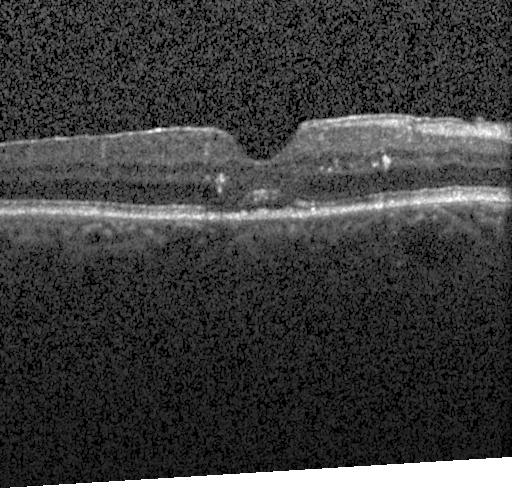

OCT line scan · spectral-domain optical coherence tomography · centered on the fovea.
Diagnosis: choroidal neovascularization.